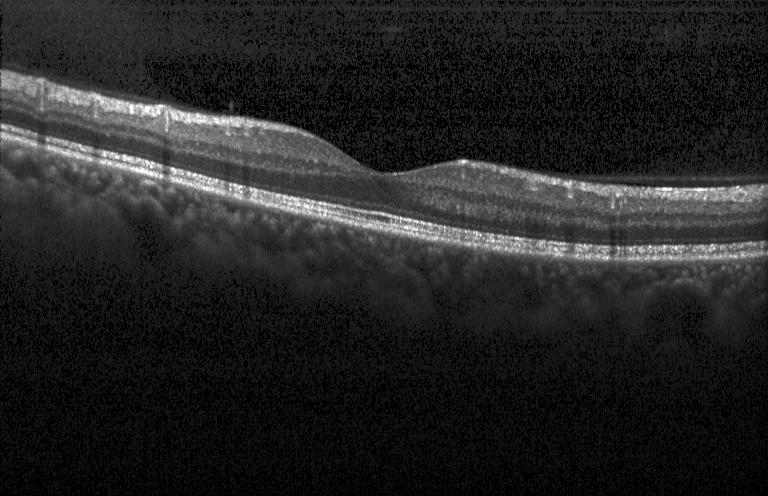

Optical coherence tomography scan, spectral-domain OCT.
Diagnosis: no choroidal neovascularization, no diabetic macular edema, and no drusen.